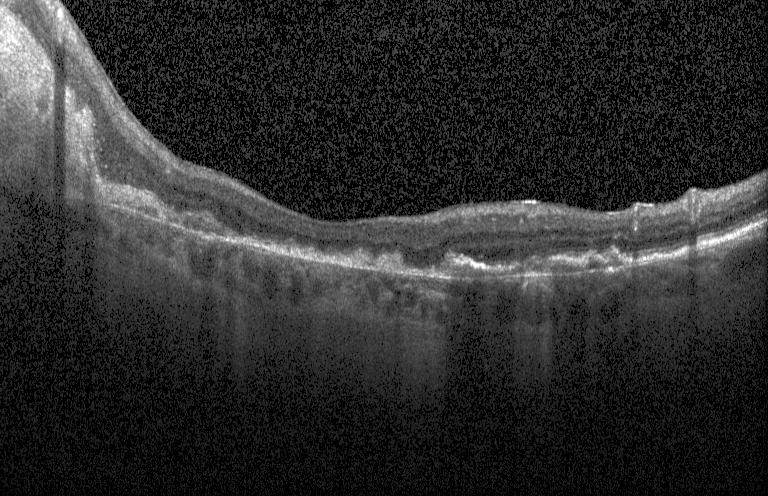

Finding: a choroidal neovascular membrane.